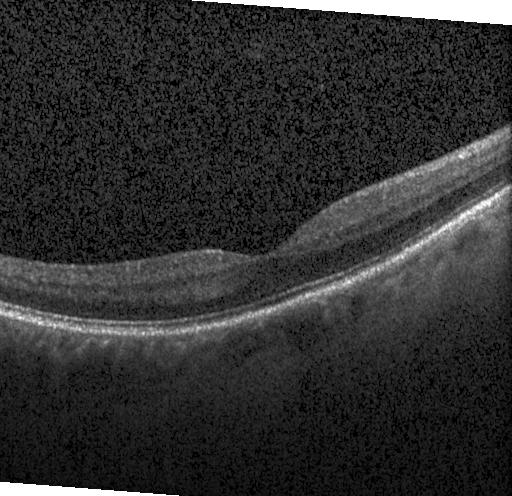
Retinal OCT cross-section. Macular scan. Impression: no CNV, no DME, and no drusen.